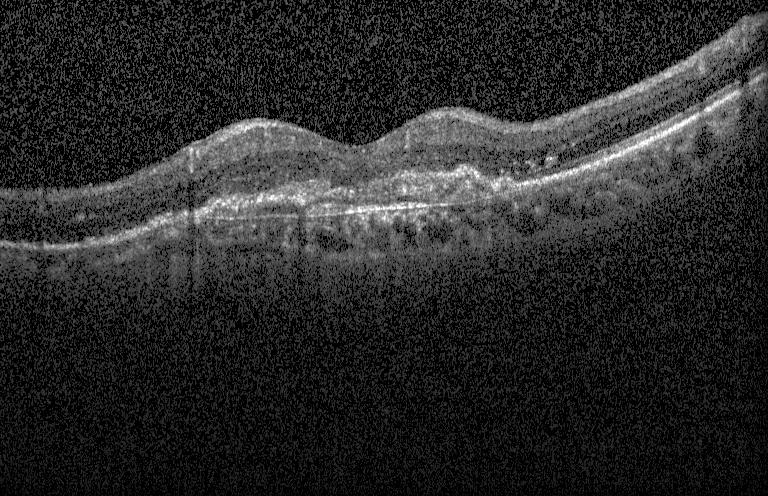 Retinal OCT B-scan. Spectral-domain OCT. OCT finding: CNV.